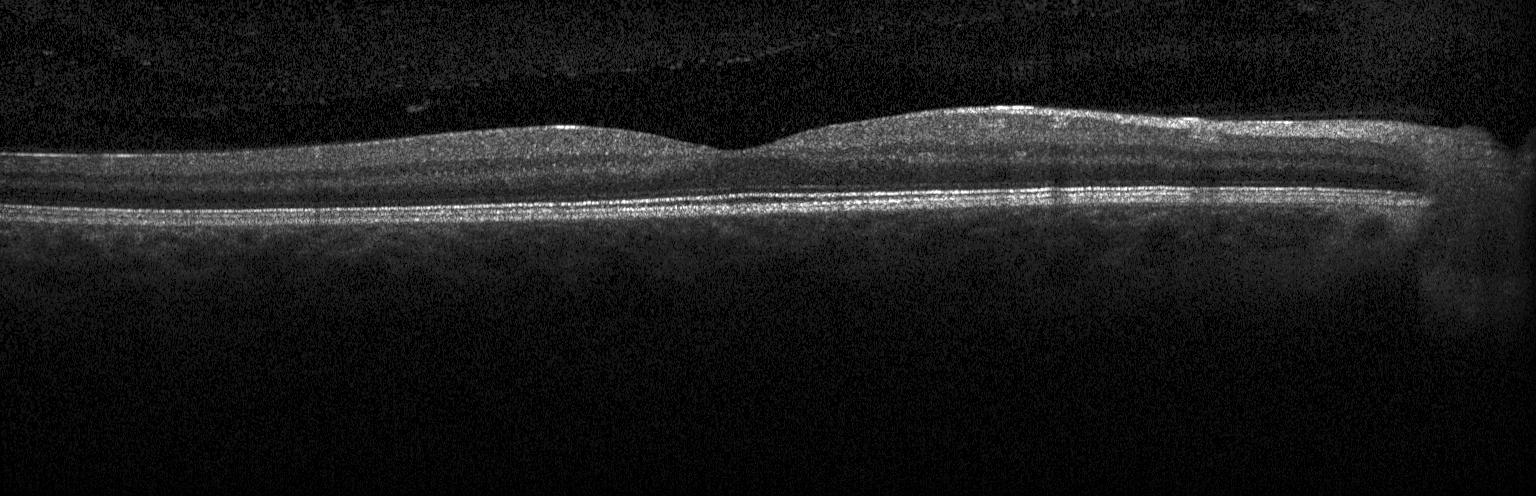 Acquired on a Heidelberg Spectralis, optical coherence tomography B-scan — Diagnosis: no evidence of CNV, DME, or drusen.